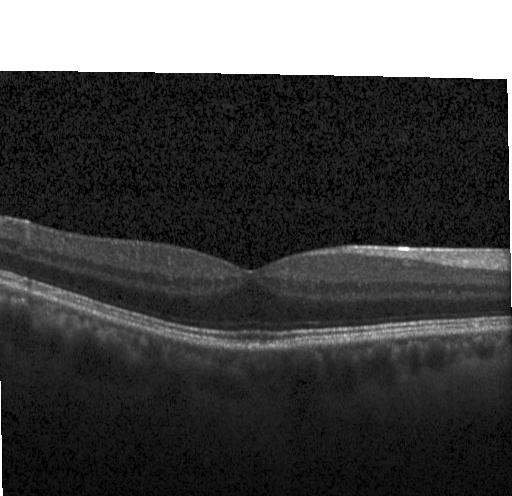
Spectral-domain OCT B-scan: neither choroidal neovascularization, diabetic macular edema, nor drusen.